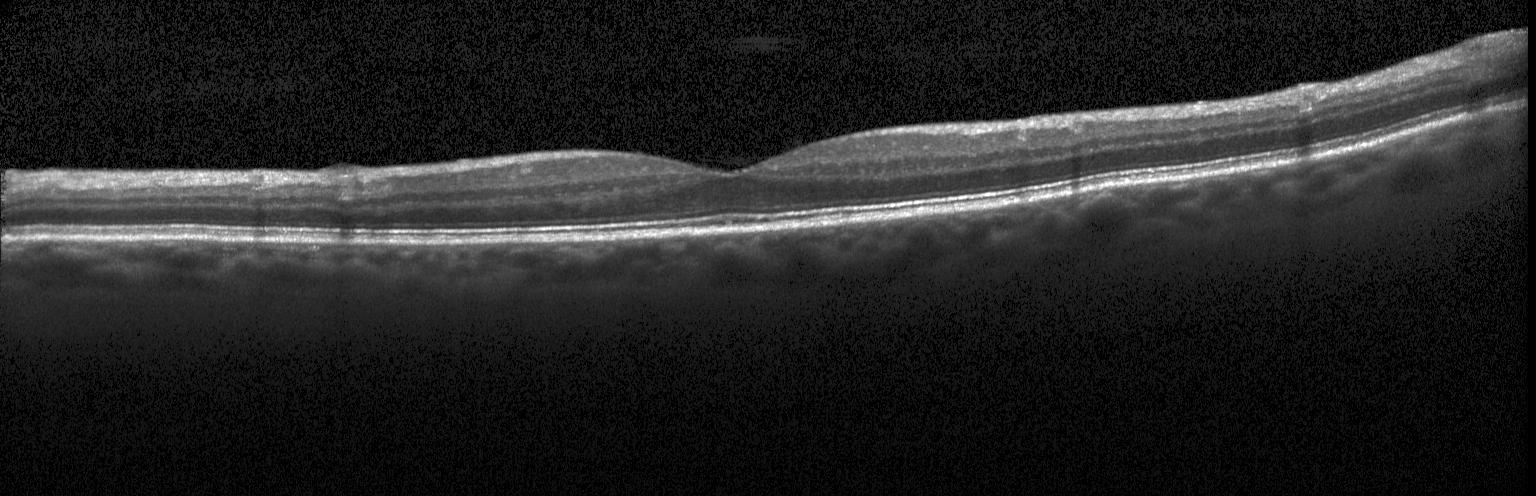 Diagnosis: no choroidal neovascularization, no diabetic macular edema, and no drusen.